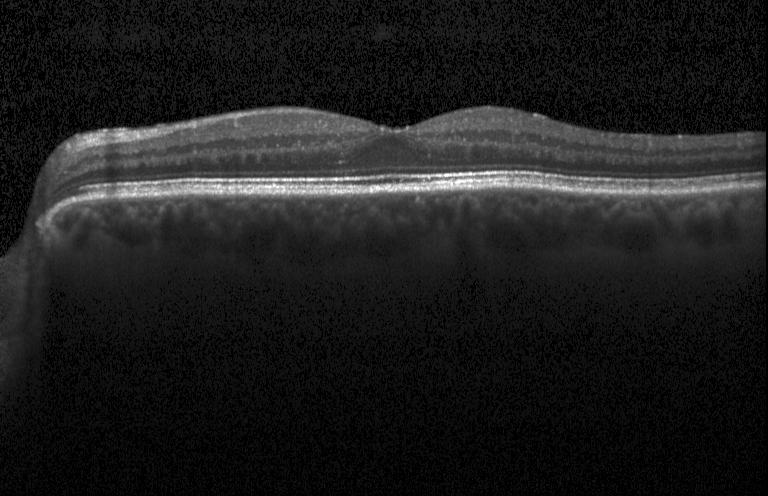 Fovea-centered · Heidelberg Spectralis OCT system · retinal OCT cross-section. Macular OCT: no choroidal neovascularization, diabetic macular edema, or drusen.